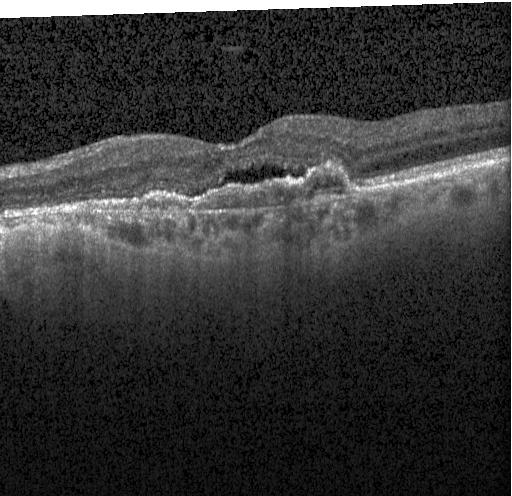 Assessment: a choroidal neovascular membrane.